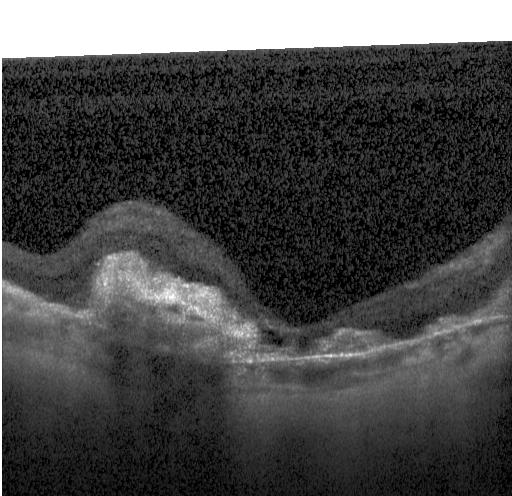

Impression: a choroidal neovascular membrane.